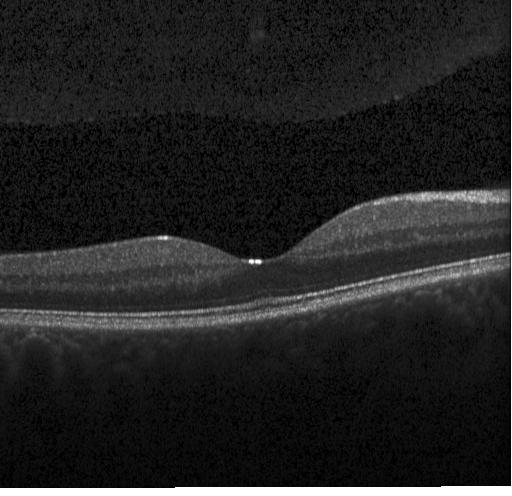
Diagnosis: no evidence of choroidal neovascularization, diabetic macular edema, or drusen.